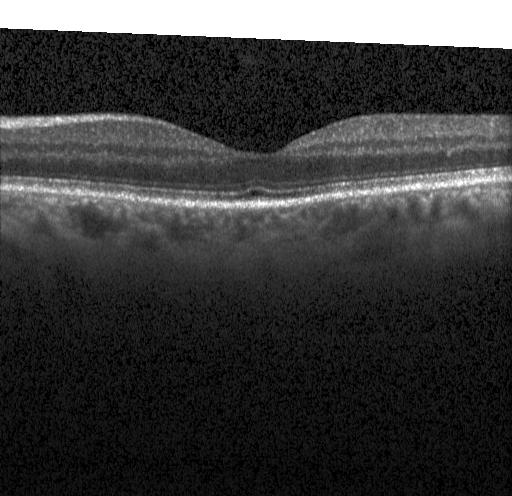

OCT B-scan; SD-OCT
OCT finding: neither CNV, DME, nor drusen.